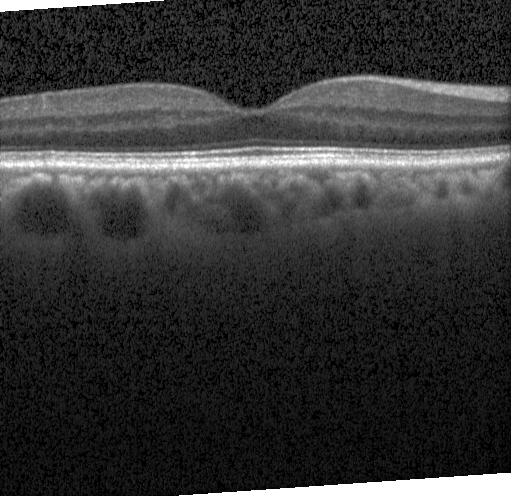 Horizontal scan through the fovea · spectral-domain optical coherence tomography · optical coherence tomography scan. Impression: no evidence of choroidal neovascularization, diabetic macular edema, or drusen.